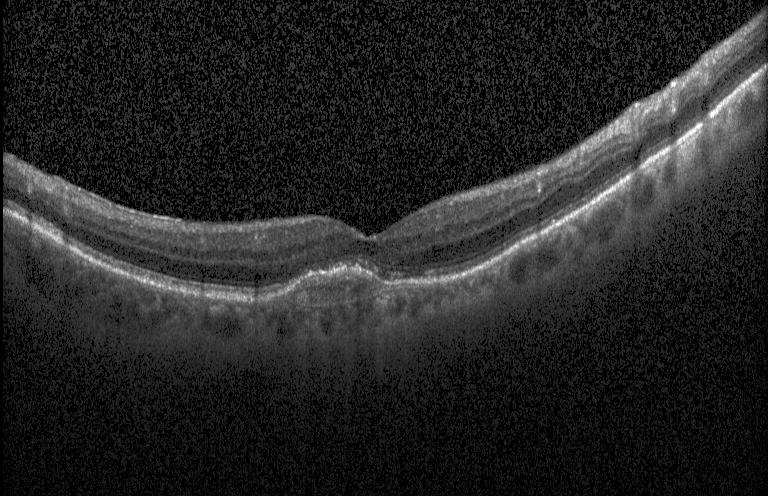

Finding: choroidal neovascularization.